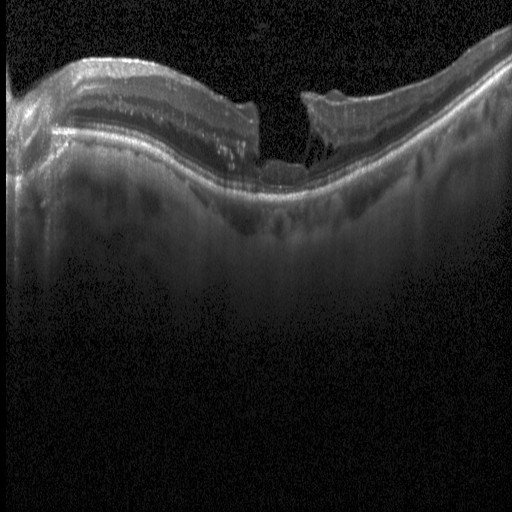
Retinal OCT cross-section.
Impression: diabetic macular edema (DME).